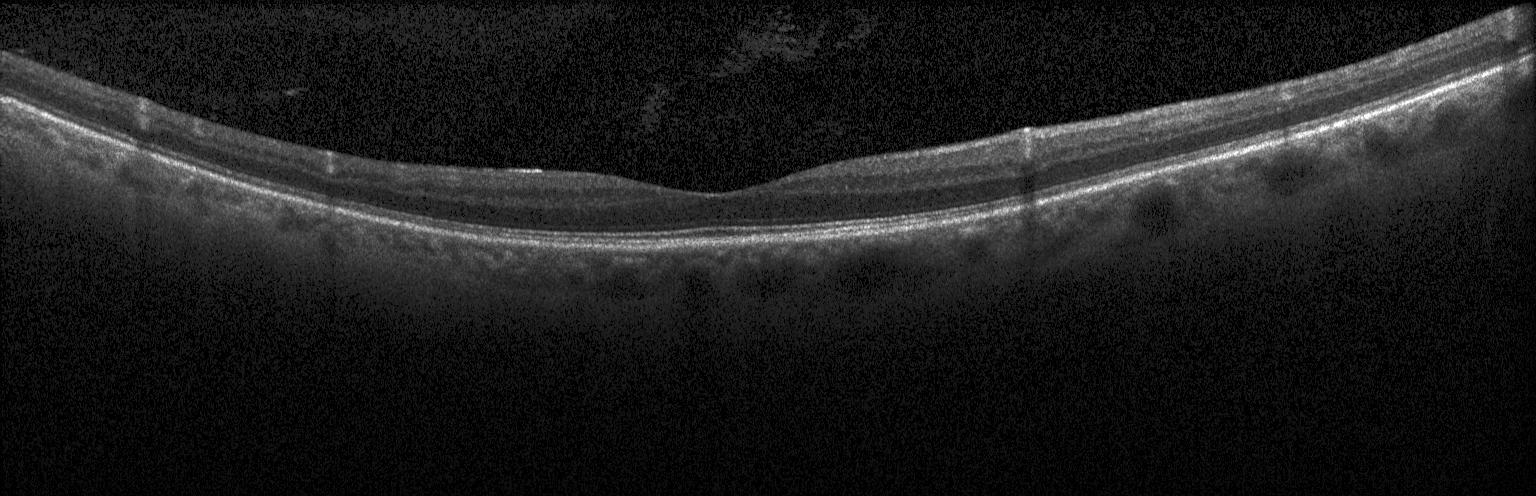
Finding: no choroidal neovascularization, diabetic macular edema, or drusen.